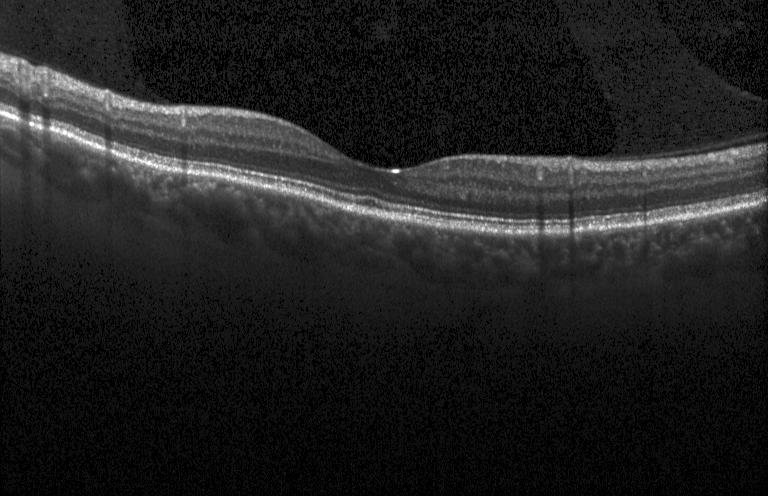

OCT finding: no choroidal neovascularization, diabetic macular edema, or drusen.